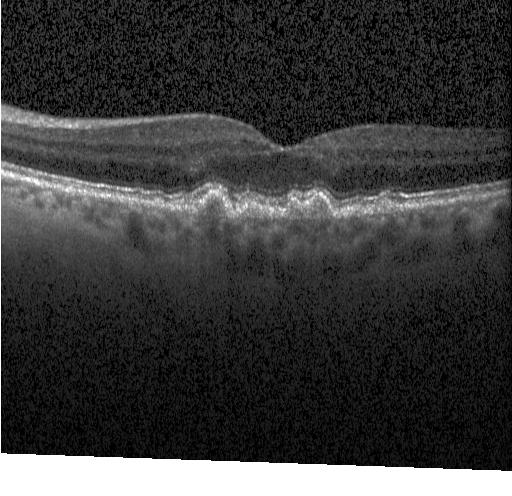

OCT B-scan; instrument: Heidelberg Spectralis
Macular OCT: sub-RPE drusenoid deposits.